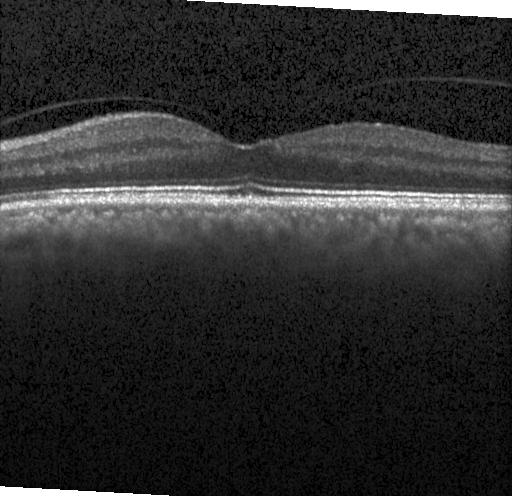 Heidelberg Spectralis. Retinal OCT cross-section.
Finding: neither choroidal neovascularization, diabetic macular edema, nor drusen.